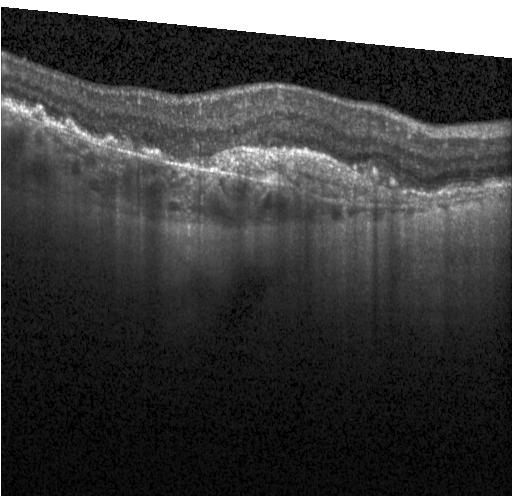
Spectral-domain optical coherence tomography; optical coherence tomography scan.
OCT finding: a choroidal neovascular membrane.